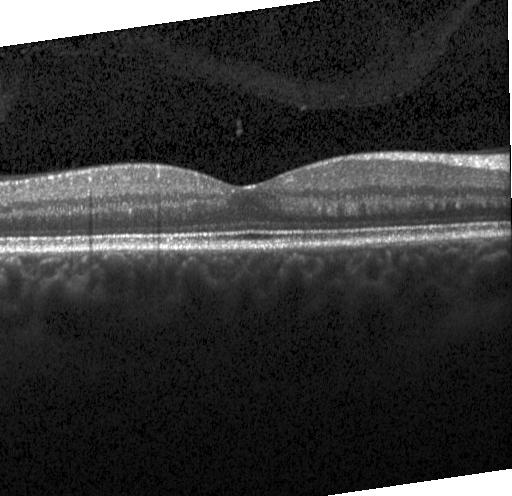 Impression: no CNV, no DME, and no drusen.